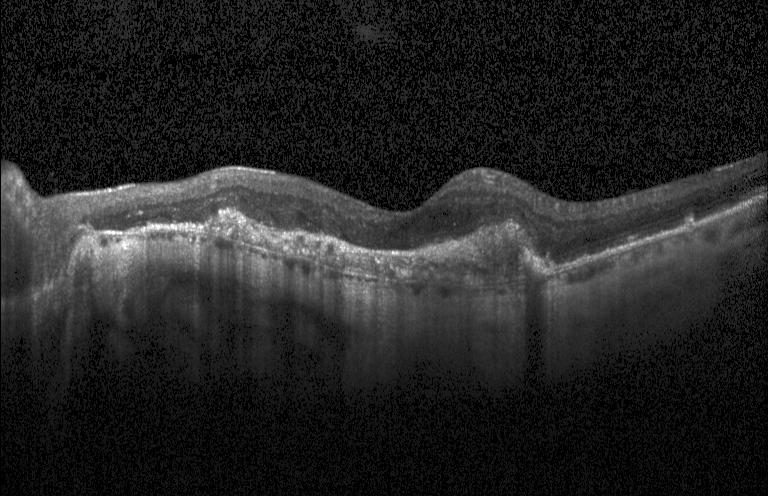
Macular OCT: CNV.